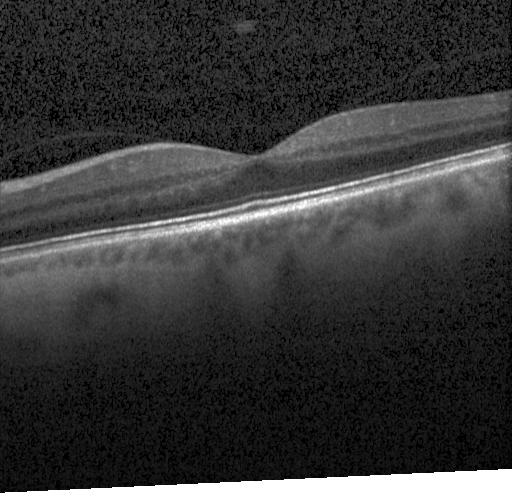
Acquired on a Heidelberg Spectralis; retinal OCT B-scan; spectral-domain optical coherence tomography.
The scan shows no evidence of choroidal neovascularization, diabetic macular edema, or drusen.